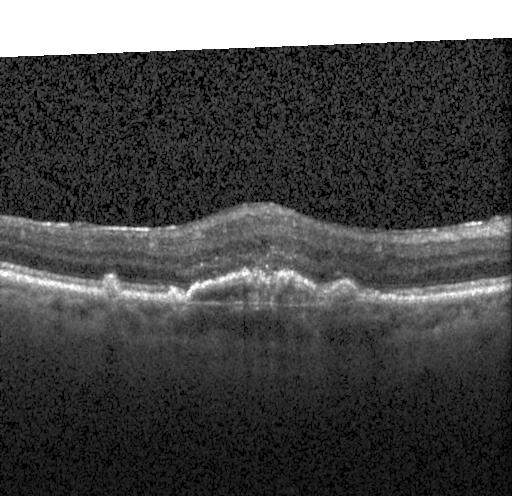
This B-scan demonstrates a choroidal neovascular membrane.